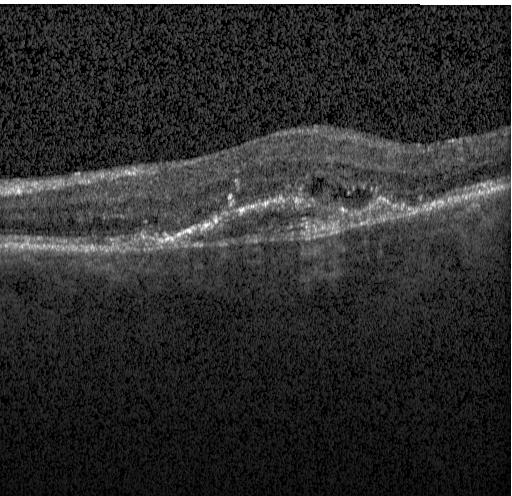
OCT B-scan showing choroidal neovascularization.